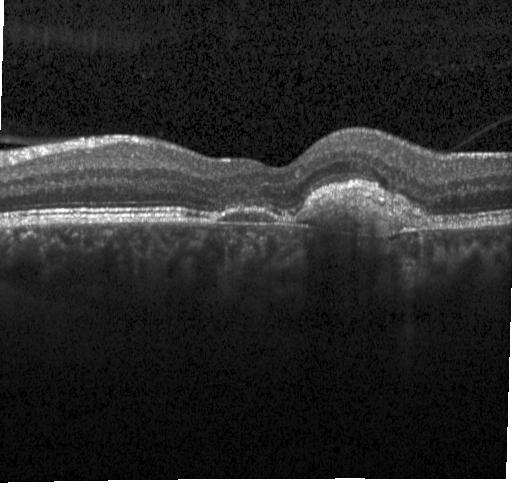

Centered on the fovea; OCT line scan. This B-scan demonstrates a choroidal neovascular membrane.